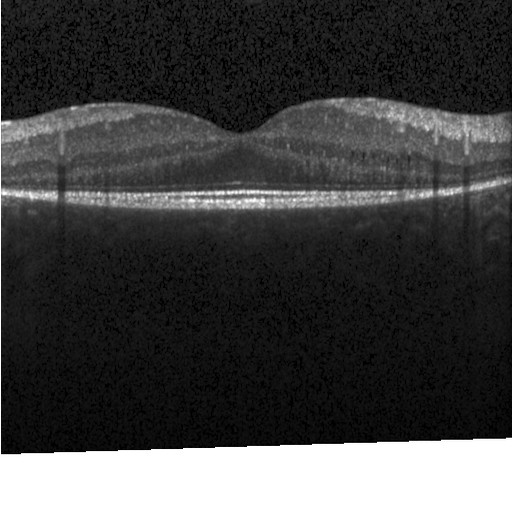 Through the macula. Optical coherence tomography B-scan. Heidelberg Spectralis — Assessment: diabetic macular edema.